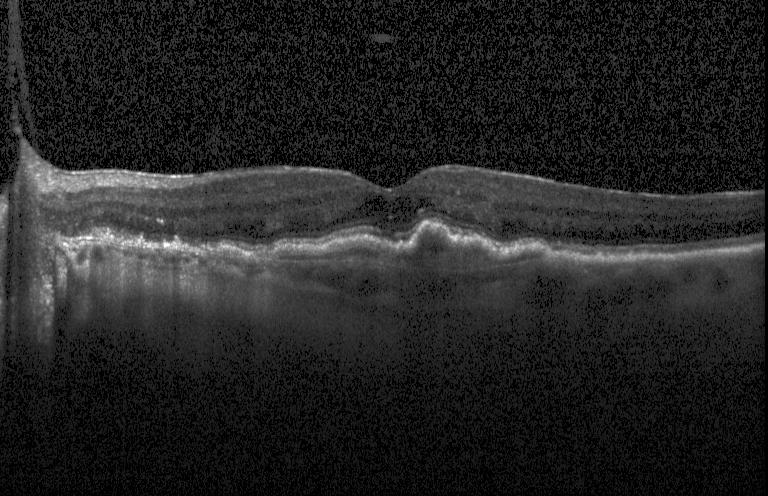

Heidelberg Spectralis OCT system. Retinal OCT B-scan.
Impression: choroidal neovascularization.